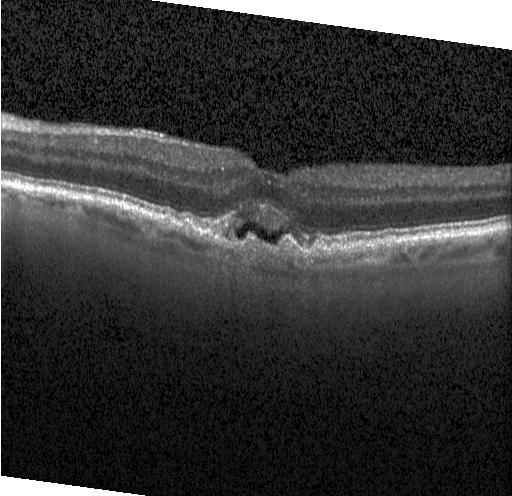 Acquired on a Heidelberg Spectralis · optical coherence tomography scan
Impression: choroidal neovascularization (CNV).